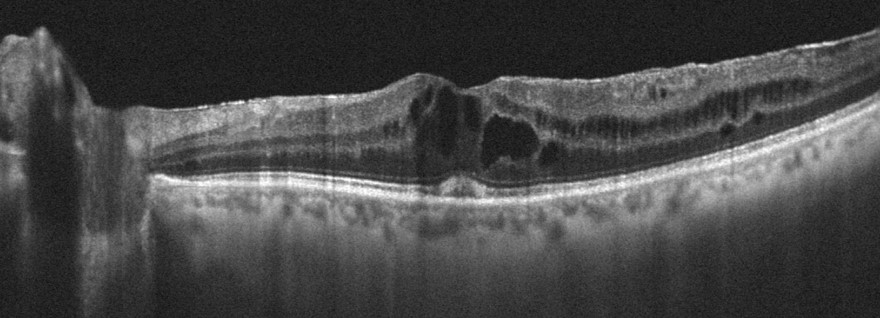
Macular scan · Optovue Avanti RTVue XR · retinal OCT cross-section. Finding: diabetic macular edema (DME).